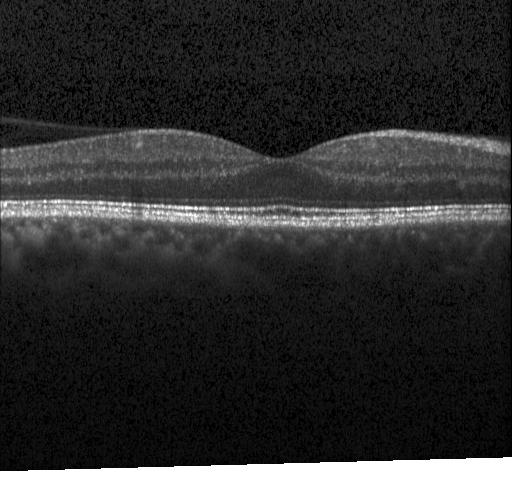

Assessment: no choroidal neovascularization, no diabetic macular edema, and no drusen.